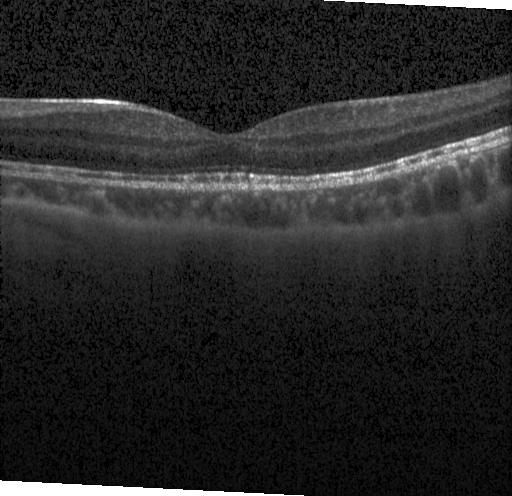 No choroidal neovascularization, diabetic macular edema, or drusen.